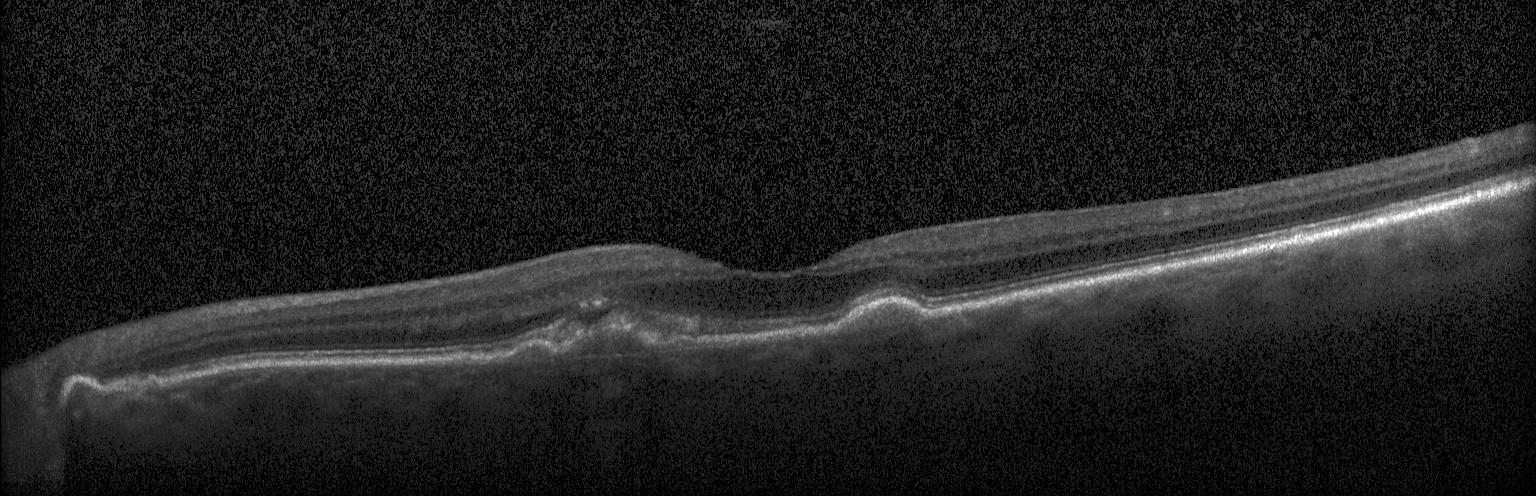 Retinal OCT B-scan — Diagnosis: a choroidal neovascular membrane.